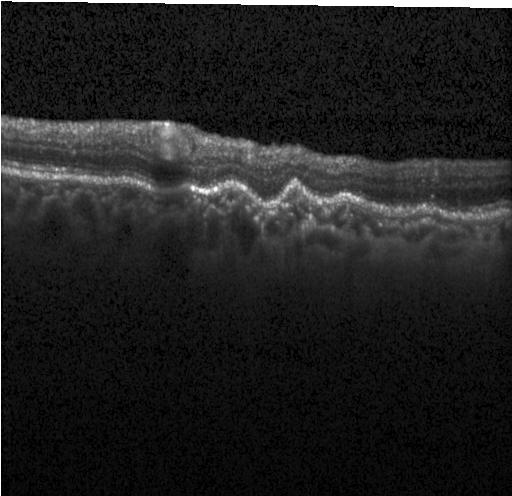
Optical coherence tomography B-scan; fovea-centered; instrument: Heidelberg Spectralis.
Finding: CNV.